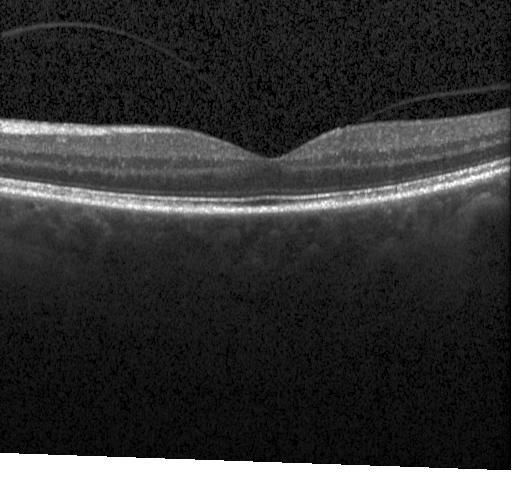

Retinal OCT B-scan, centered on the fovea
The scan shows neither choroidal neovascularization, diabetic macular edema, nor drusen.